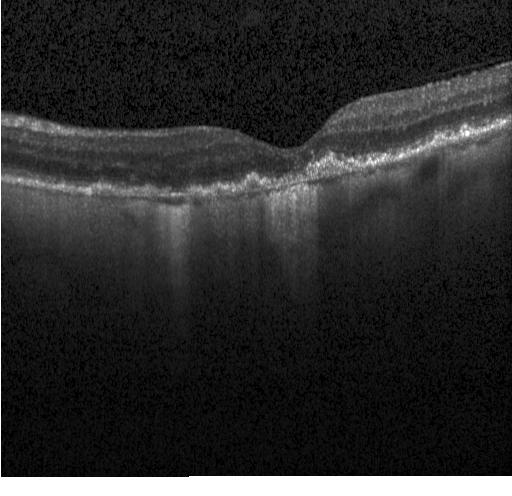 Instrument: Heidelberg Spectralis · through the macula · optical coherence tomography B-scan.
Impression: a choroidal neovascular membrane.